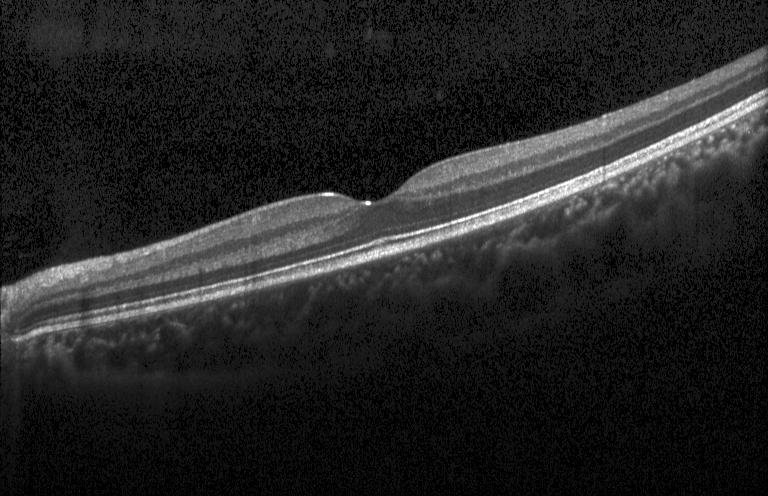
Impression: no choroidal neovascularization, diabetic macular edema, or drusen.